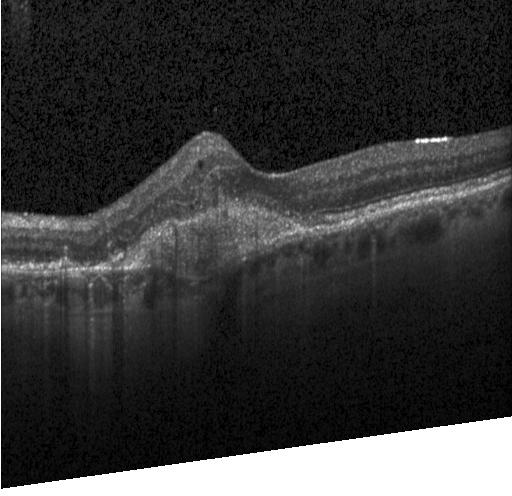
Acquired on a Heidelberg Spectralis. Optical coherence tomography scan. SD-OCT.
Choroidal neovascularization.